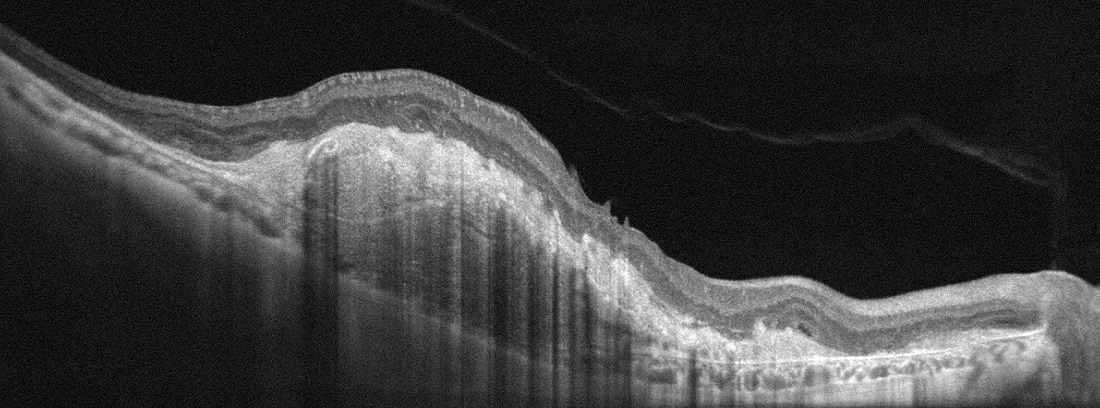 OCT B-scan showing AMD.